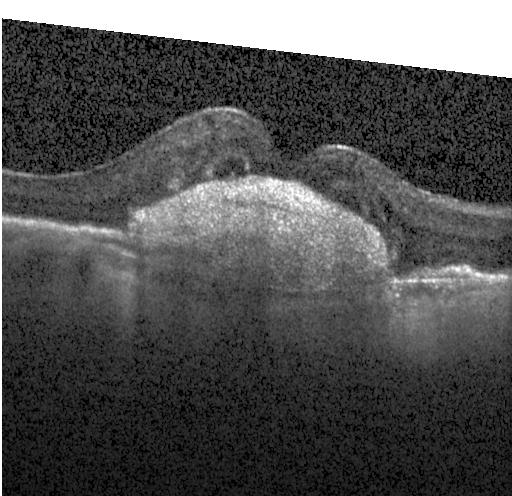

Diagnosis: choroidal neovascularization (CNV).